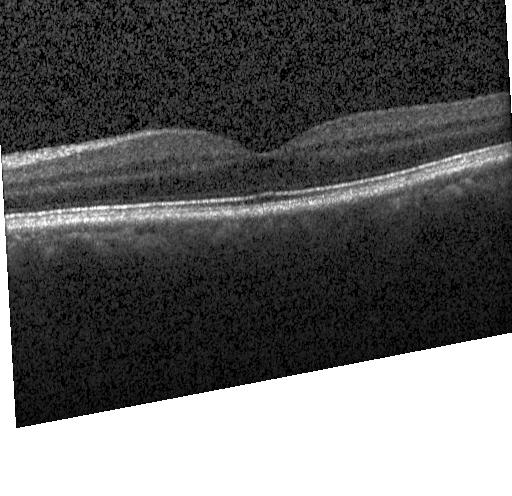 Diagnosis: no choroidal neovascularization, no diabetic macular edema, and no drusen.